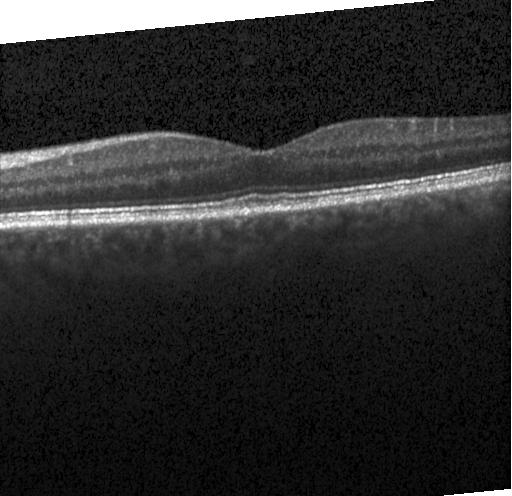 Spectral-domain OCT · retinal OCT cross-section · centered on the fovea · instrument: Heidelberg Spectralis. This B-scan demonstrates no evidence of choroidal neovascularization, diabetic macular edema, or drusen.